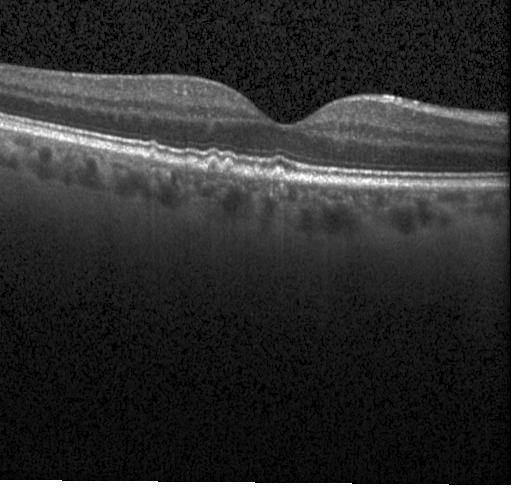

Optical coherence tomography B-scan
Sub-RPE drusenoid deposits.